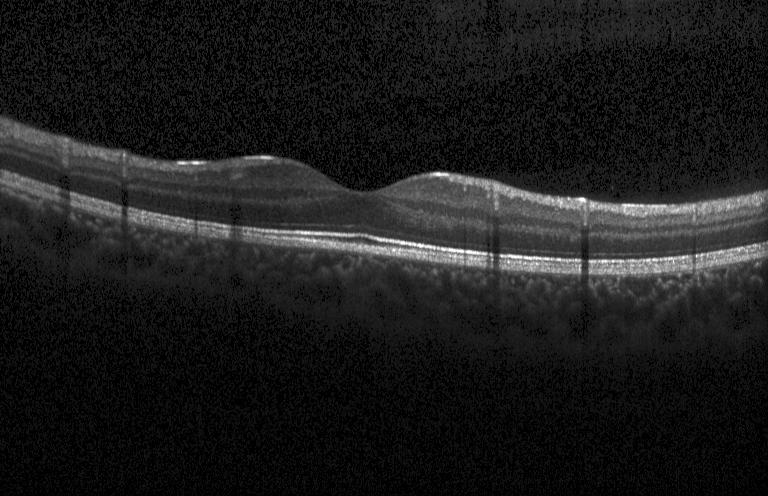
Optical coherence tomography B-scan — No CNV, DME, or drusen.